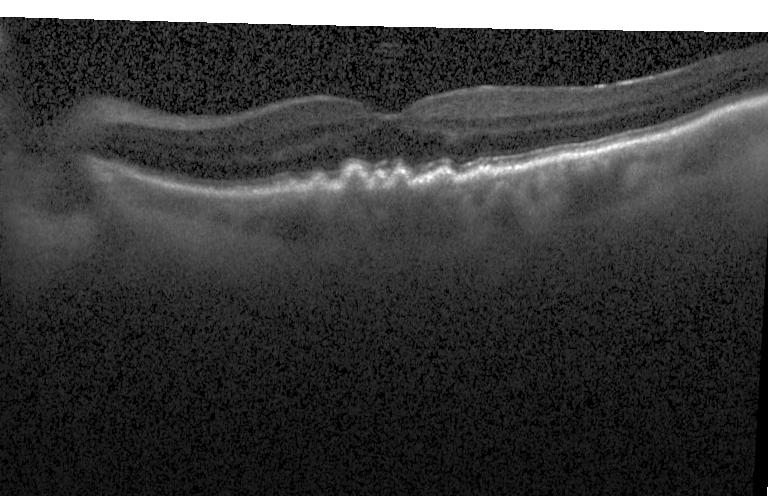 OCT B-scan. Through the macula. SD-OCT. Instrument: Heidelberg Spectralis
Sub-RPE drusenoid deposits.